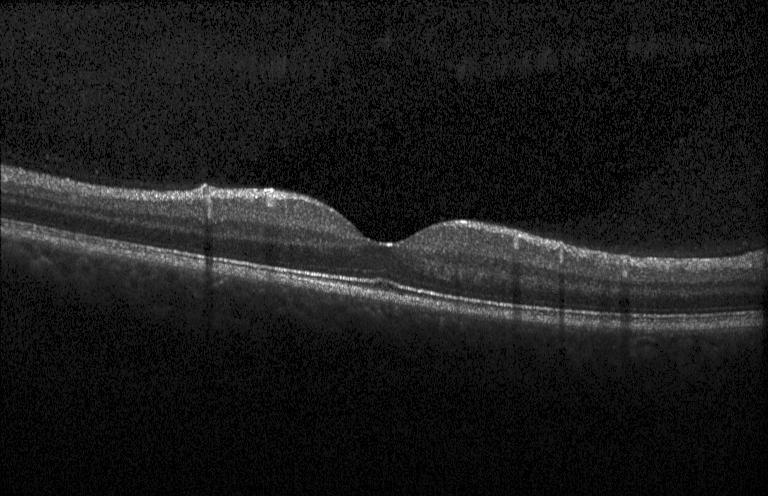

Optical coherence tomography scan, Heidelberg Spectralis. This B-scan demonstrates no choroidal neovascularization, diabetic macular edema, or drusen.